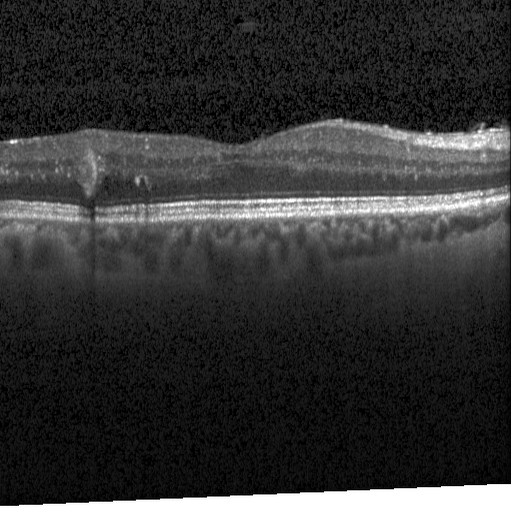
Optical coherence tomography scan · spectral-domain OCT.
OCT finding: diabetic macular edema.